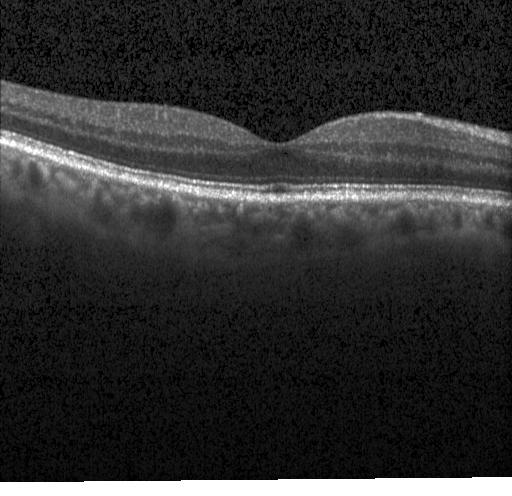 Retinal OCT B-scan.
Impression: no CNV, no DME, and no drusen.